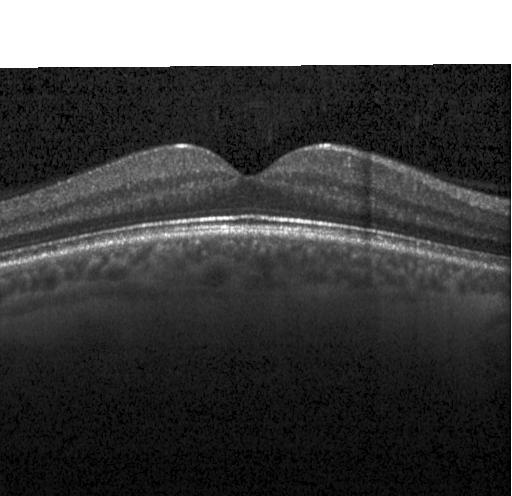
This B-scan demonstrates no CNV, no DME, and no drusen.